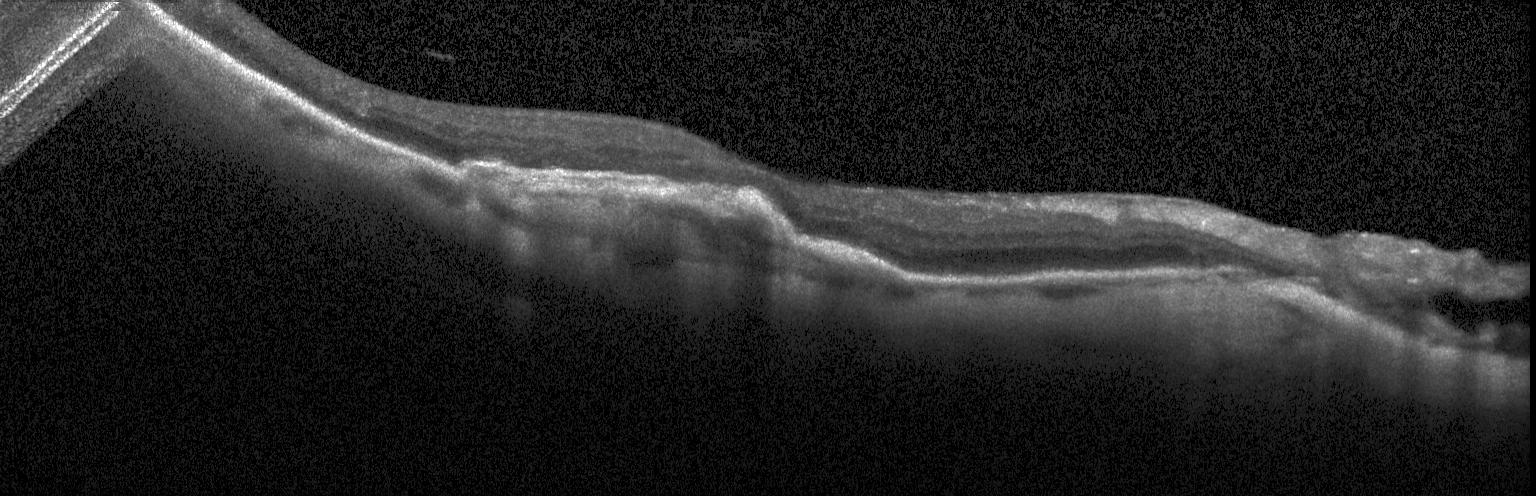
Finding: a choroidal neovascular membrane.